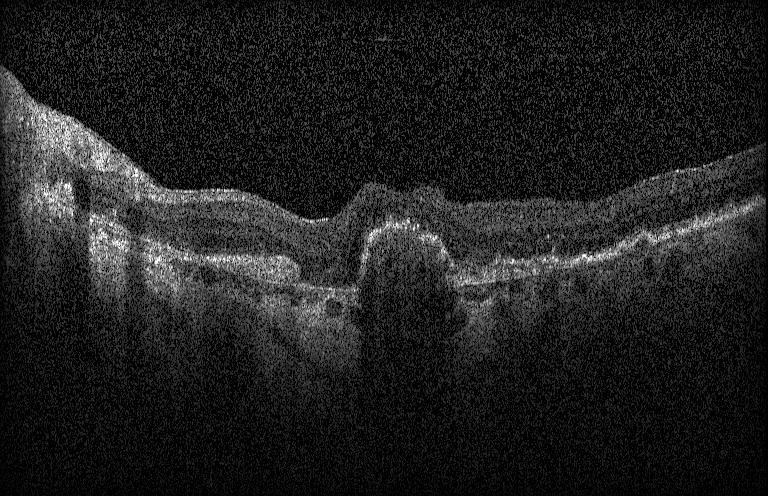 Impression: a choroidal neovascular membrane.